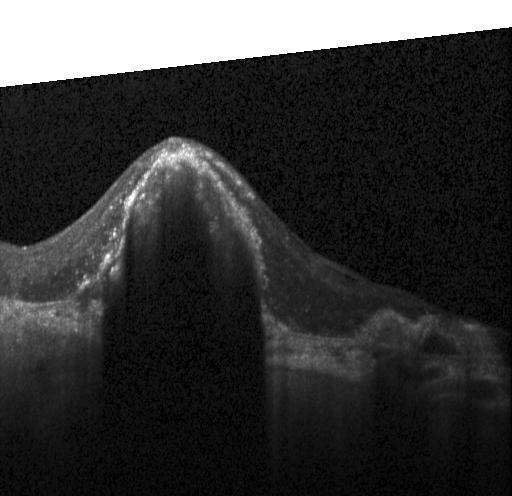 Finding: a choroidal neovascular membrane.